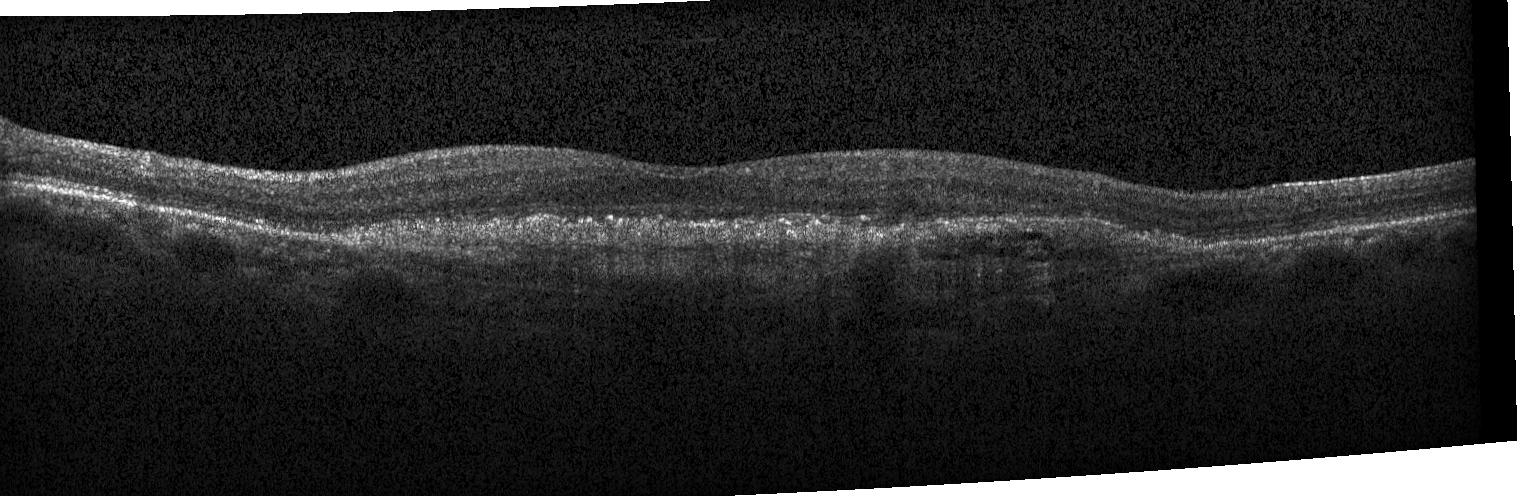 OCT B-scan
Choroidal neovascularization (CNV).